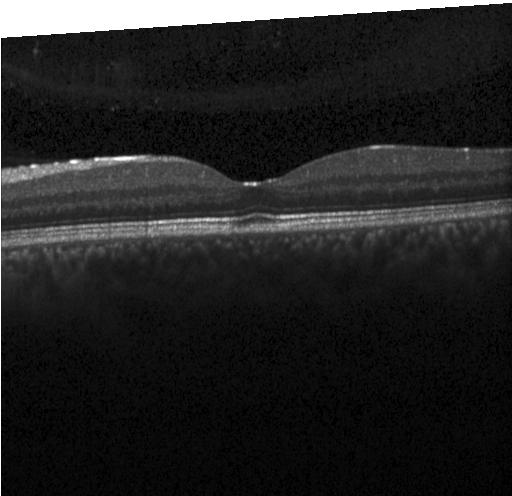 Finding: no evidence of choroidal neovascularization, diabetic macular edema, or drusen.